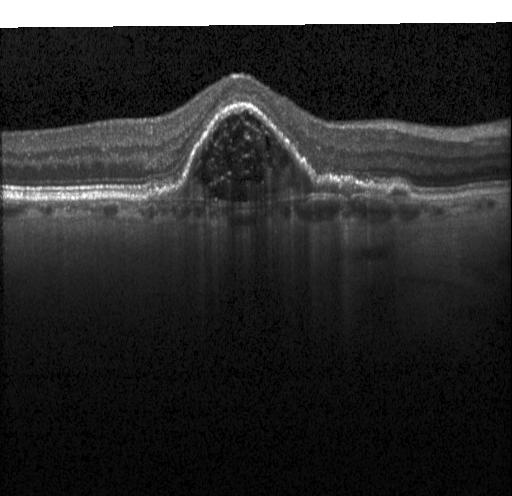
SD-OCT; instrument: Heidelberg Spectralis; centered on the fovea; retinal OCT B-scan.
Finding: a choroidal neovascular membrane.